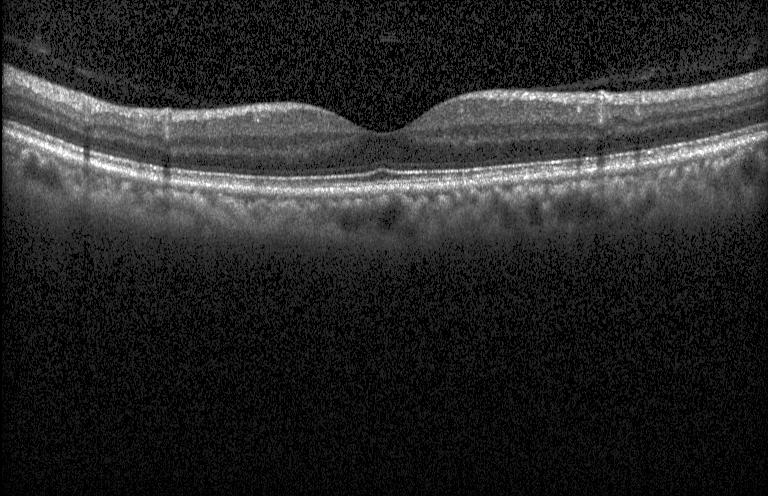

Acquired on a Heidelberg Spectralis. Retinal OCT B-scan. Spectral-domain OCT. Fovea-centered.
No choroidal neovascularization, diabetic macular edema, or drusen.